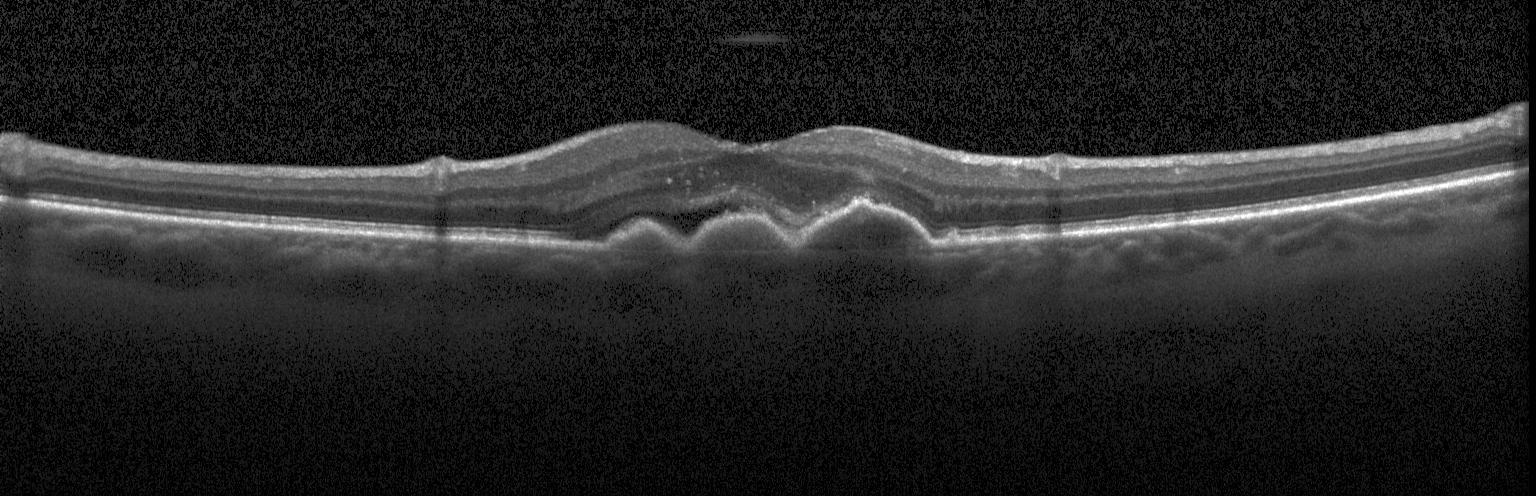

Centered on the fovea. Retinal OCT cross-section
This B-scan demonstrates choroidal neovascularization.